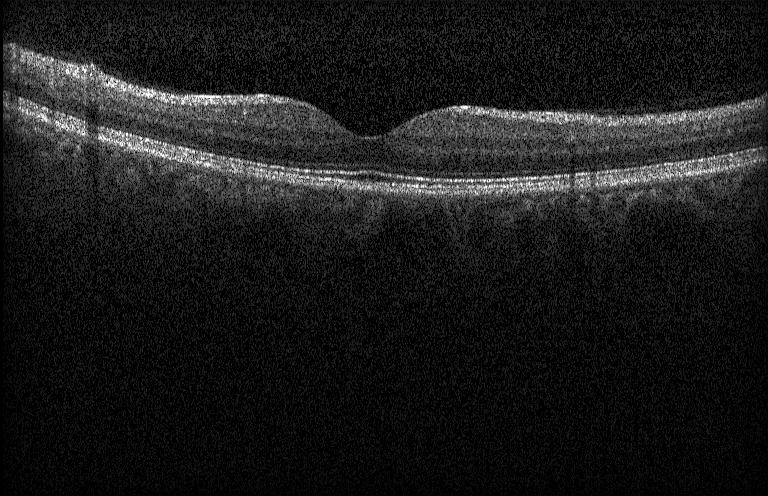
OCT line scan
OCT finding: no evidence of choroidal neovascularization, diabetic macular edema, or drusen.